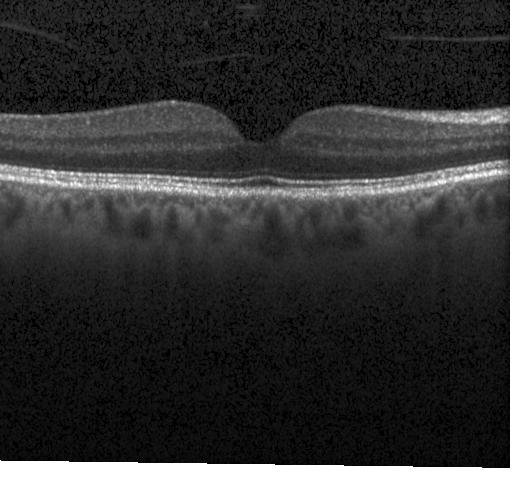 Macular scan; Heidelberg Spectralis; OCT line scan. No CNV, no DME, and no drusen.